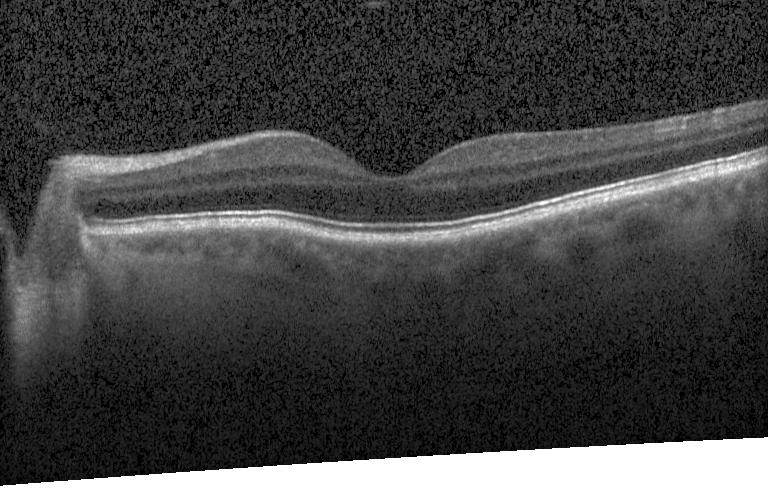
Diagnosis: no CNV, no DME, and no drusen.